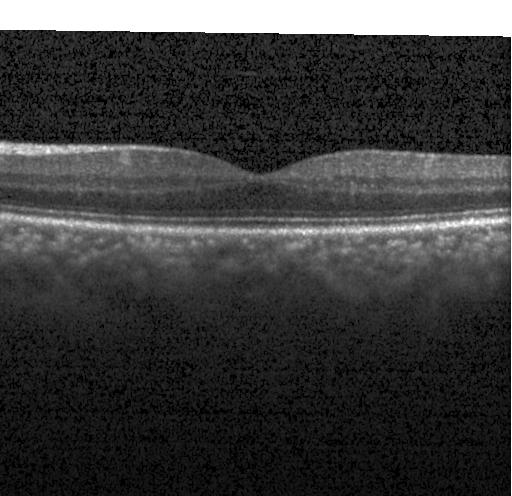
Fovea-centered, optical coherence tomography B-scan. Diagnosis: no CNV, DME, or drusen.